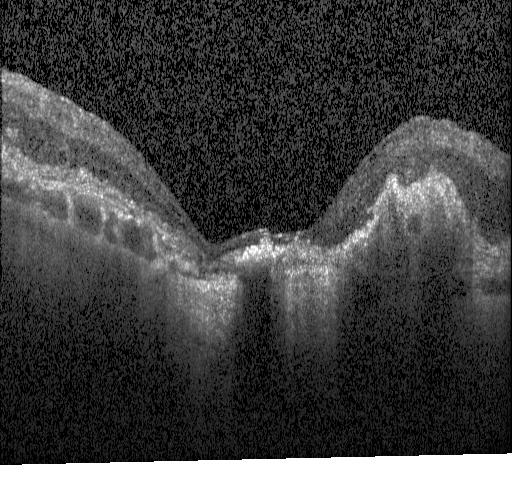 This B-scan demonstrates a choroidal neovascular membrane.